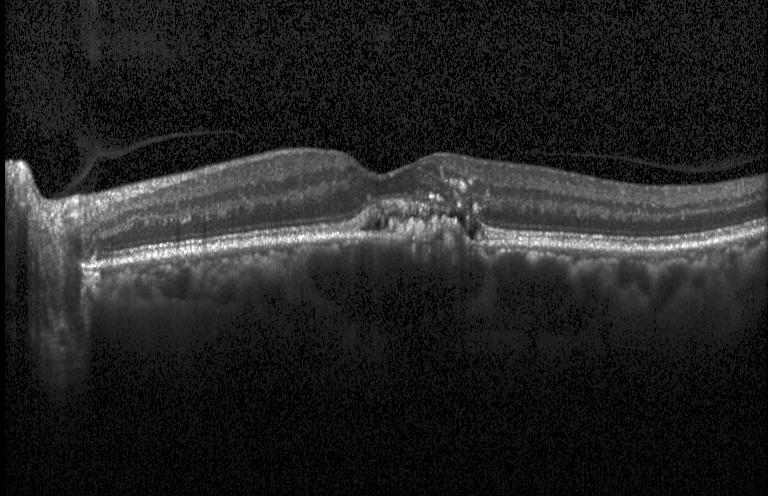
Retinal OCT cross-section showing choroidal neovascularization (CNV).